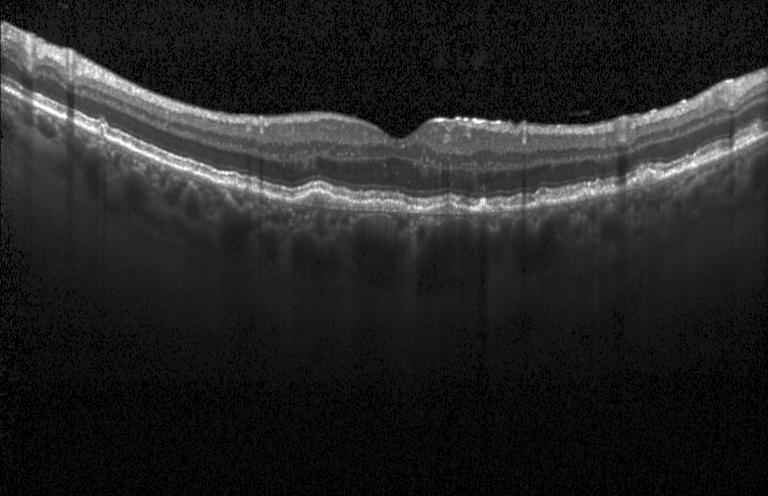
Finding: a choroidal neovascular membrane.